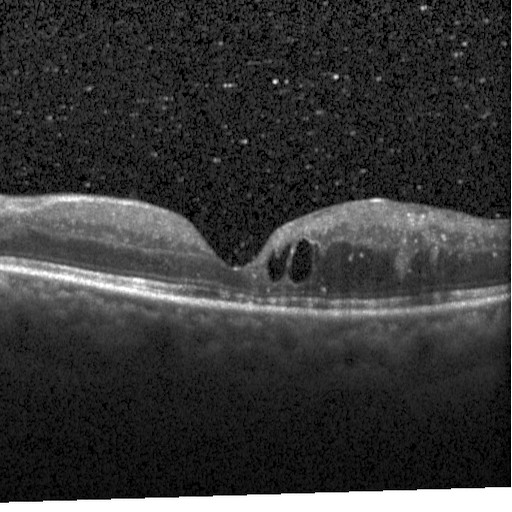

OCT finding: DME.